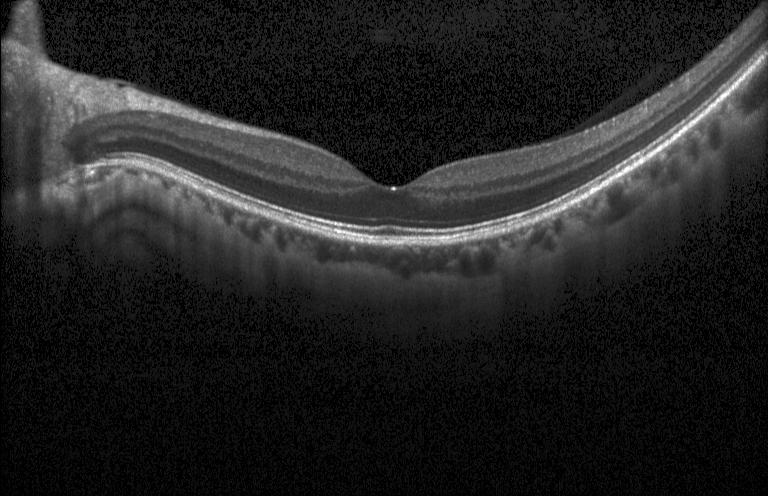

OCT B-scan.
Finding: no CNV, DME, or drusen.